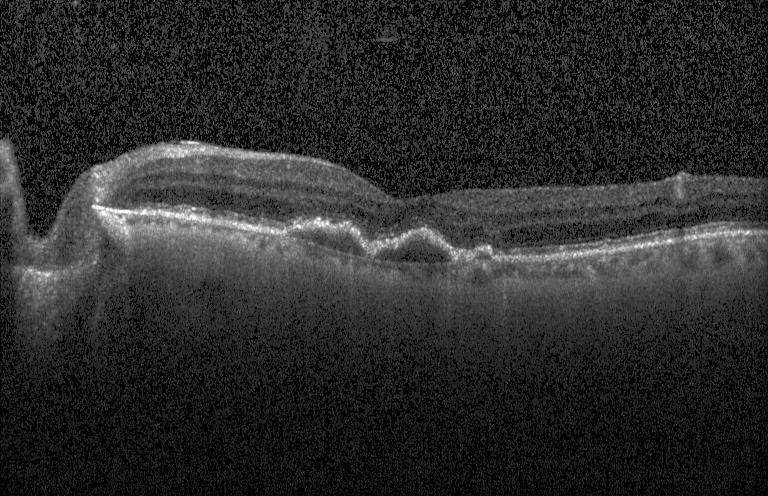
The scan shows choroidal neovascularization.